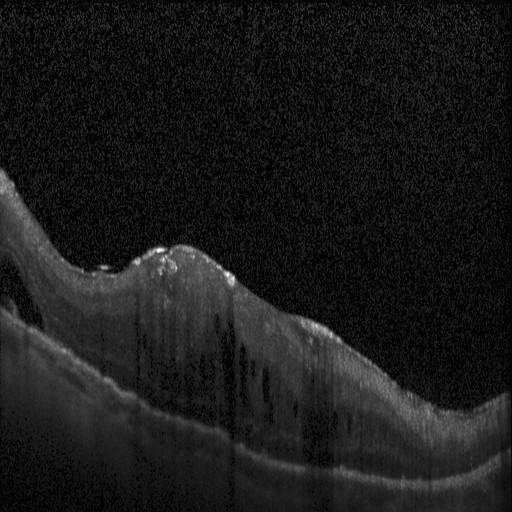 Optical coherence tomography scan. Acquired on a Heidelberg Spectralis. Spectral-domain OCT — OCT finding: diabetic macular edema (DME).